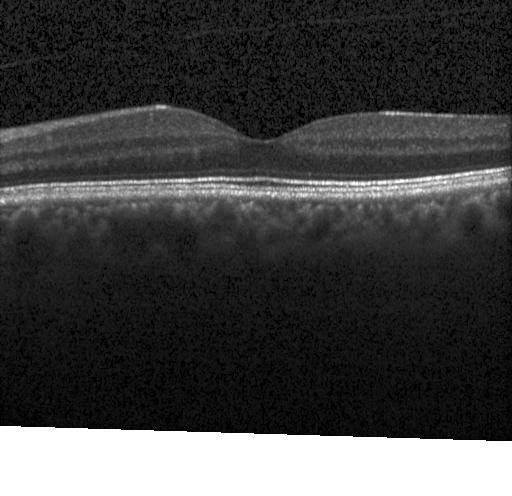
Dx: no choroidal neovascularization, no diabetic macular edema, and no drusen.